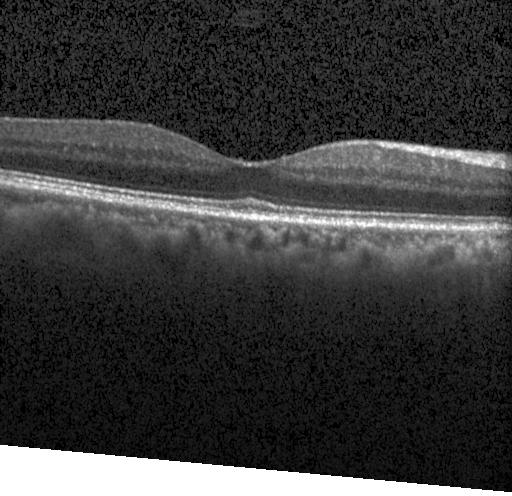
Finding: no CNV, DME, or drusen.